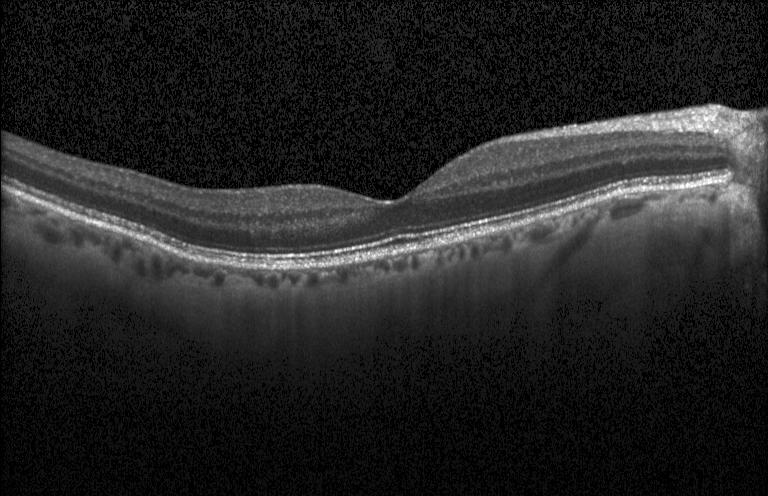
This B-scan demonstrates no choroidal neovascularization, no diabetic macular edema, and no drusen.